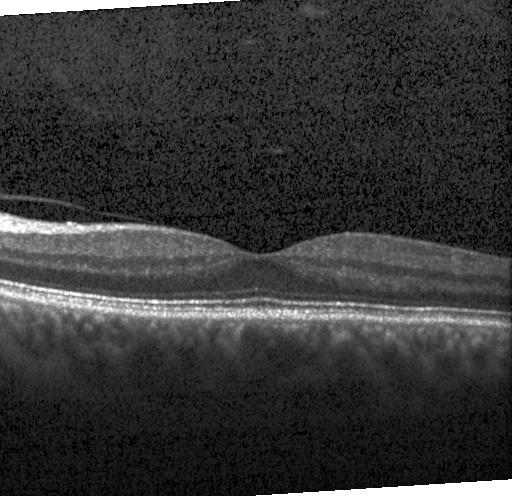 Retinal OCT B-scan; fovea-centered; SD-OCT. Dx: neither choroidal neovascularization, diabetic macular edema, nor drusen.